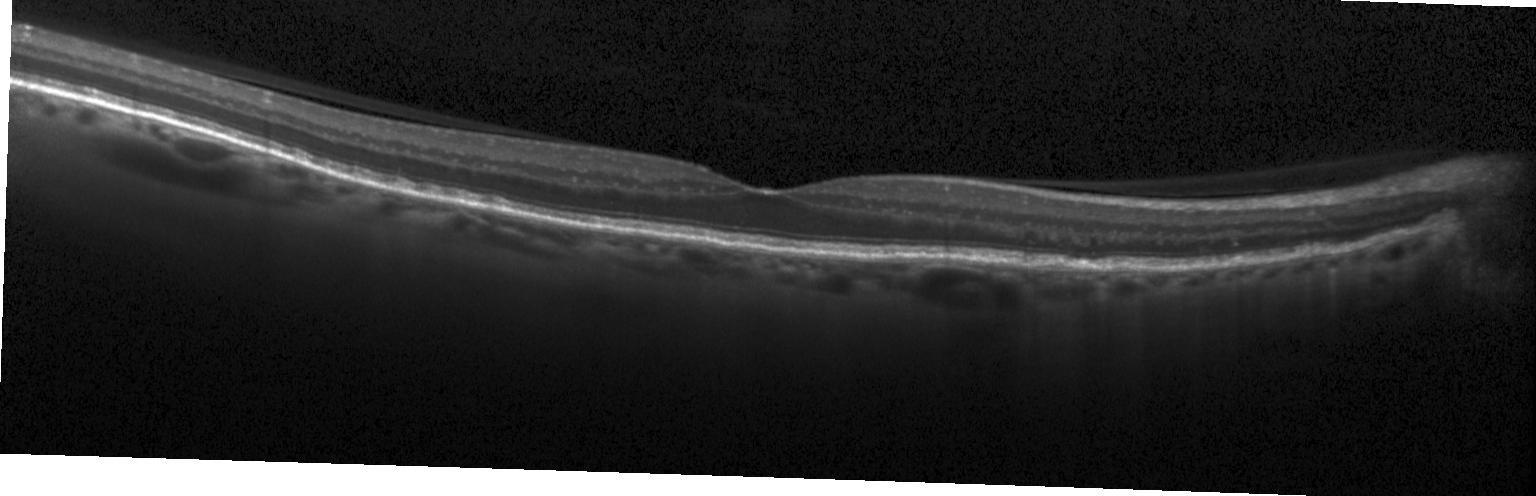
OCT line scan · Heidelberg Spectralis OCT system
The scan shows no CNV, DME, or drusen.